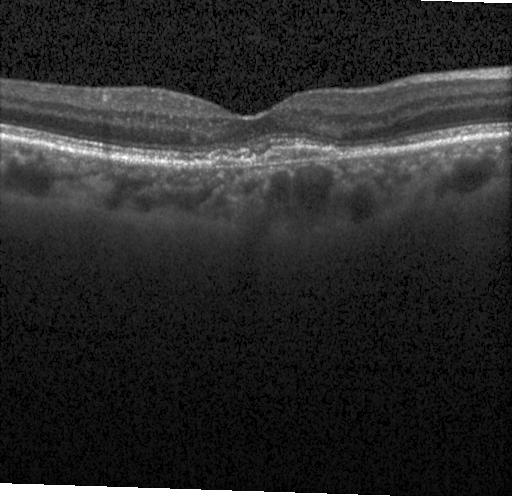 SD-OCT · retinal OCT cross-section. Finding: a choroidal neovascular membrane.